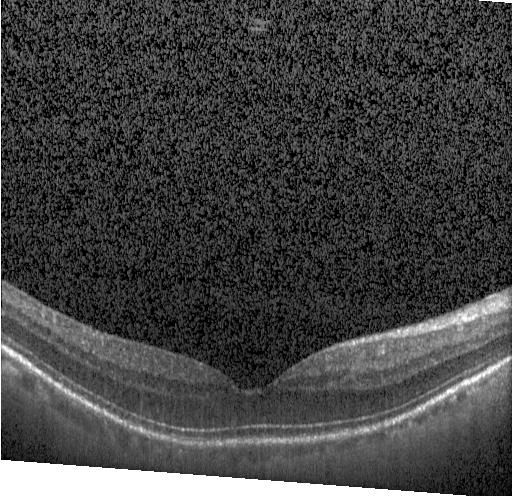 Retinal OCT B-scan · instrument: Heidelberg Spectralis
Impression: no choroidal neovascularization, no diabetic macular edema, and no drusen.